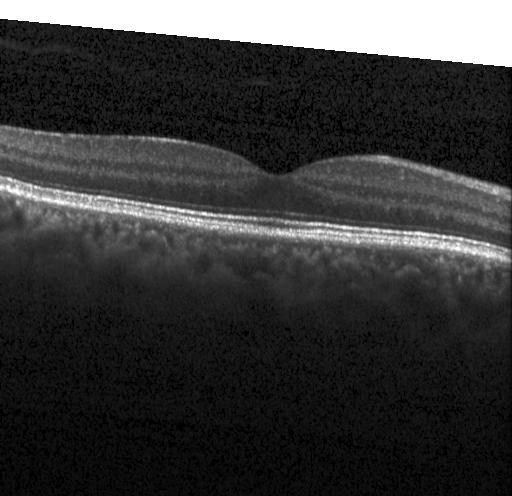

Retinal OCT B-scan — Diagnosis: no choroidal neovascularization, no diabetic macular edema, and no drusen.